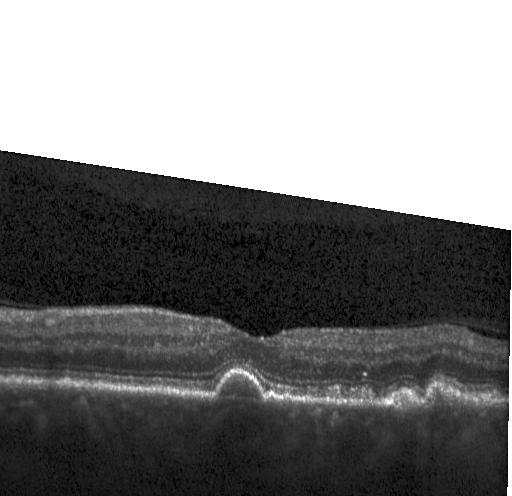

Optical coherence tomography B-scan — Assessment: multiple drusen.